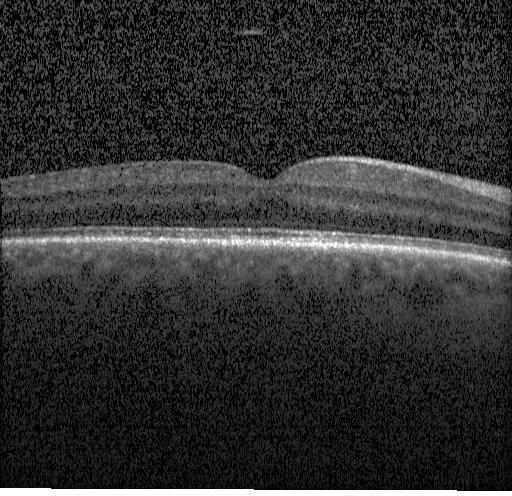
Fovea-centered · acquired on a Heidelberg Spectralis · spectral-domain OCT · OCT line scan — Assessment: no choroidal neovascularization, diabetic macular edema, or drusen.